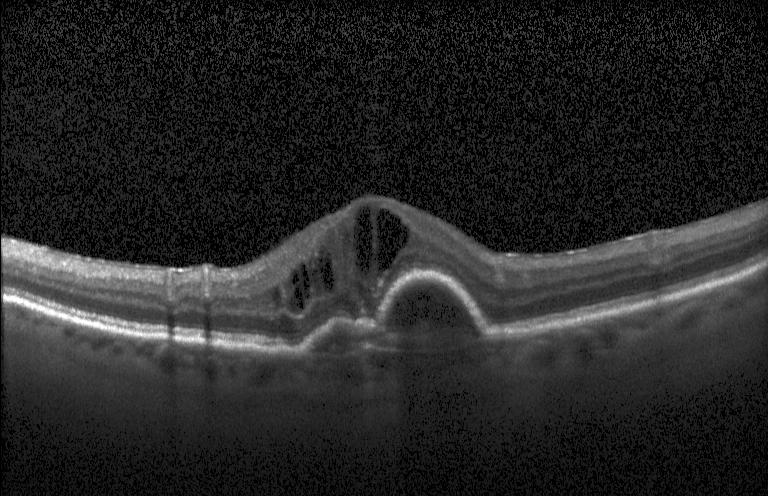
Spectral-domain optical coherence tomography · Heidelberg Spectralis · OCT B-scan — This B-scan demonstrates a choroidal neovascular membrane.